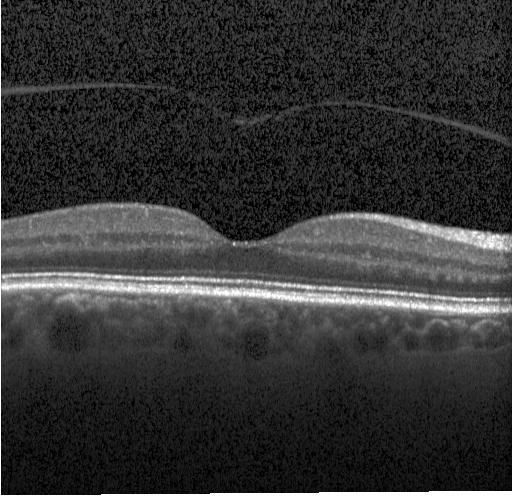
Retinal OCT cross-section showing neither choroidal neovascularization, diabetic macular edema, nor drusen.